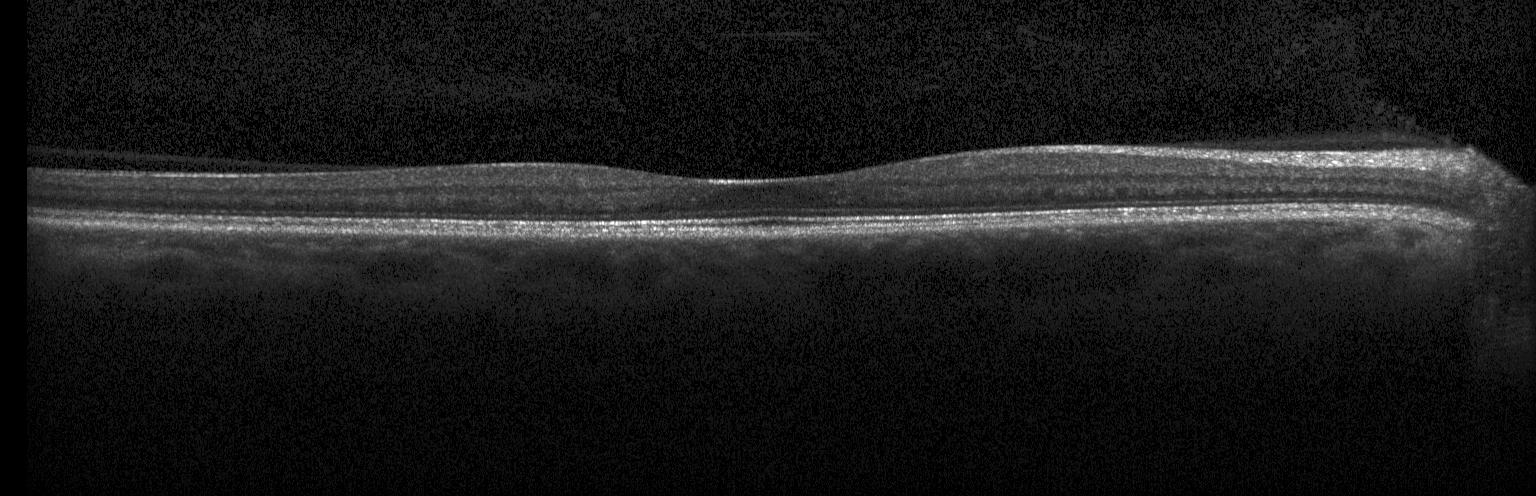
Macular scan. OCT line scan. Heidelberg Spectralis. Spectral-domain OCT.
OCT finding: no choroidal neovascularization, diabetic macular edema, or drusen.